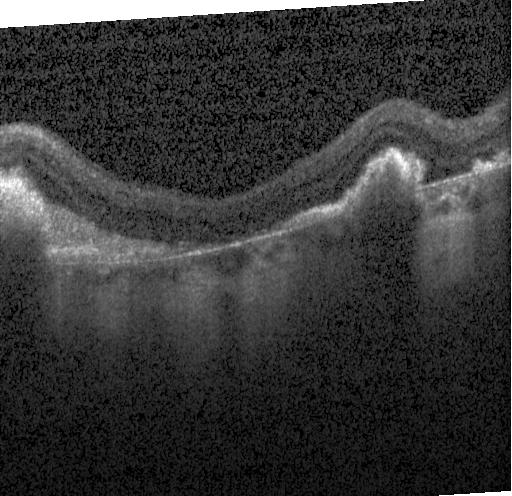 Retinal OCT cross-section — OCT finding: choroidal neovascularization.